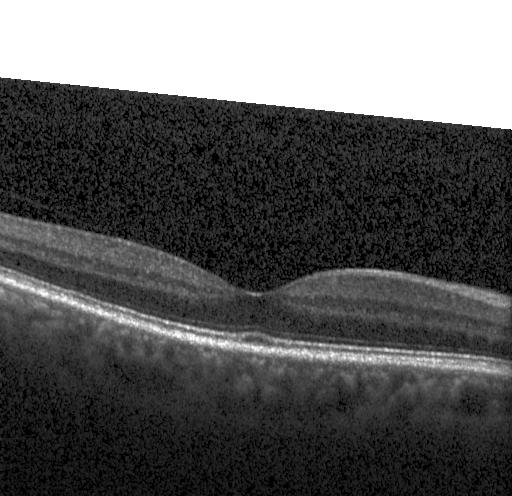
Retinal OCT cross-section showing no CNV, DME, or drusen.